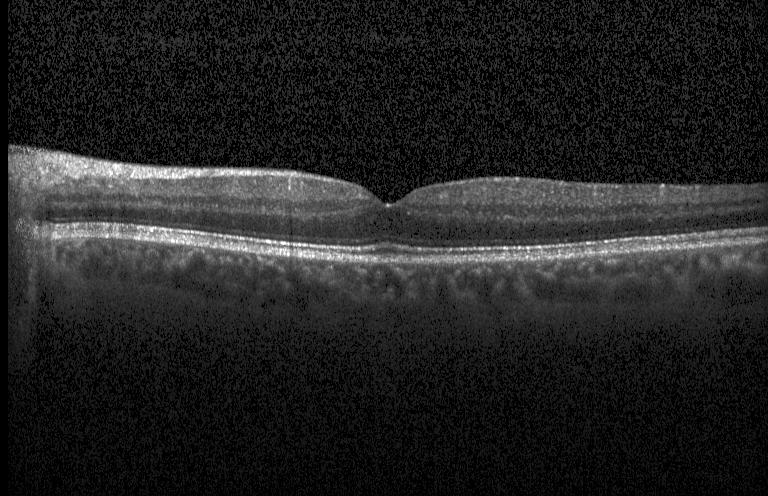
Impression: no evidence of CNV, DME, or drusen.